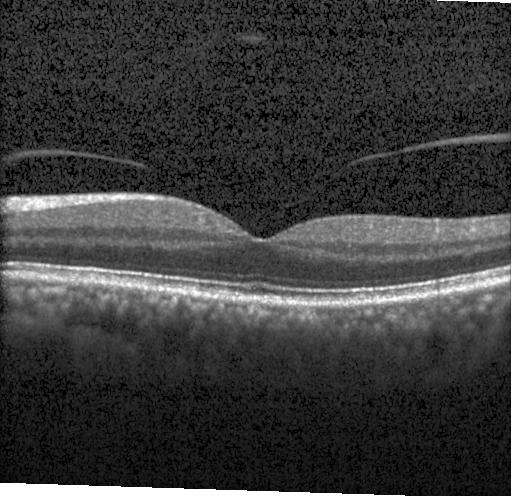

OCT line scan · spectral-domain OCT — Dx: no evidence of choroidal neovascularization, diabetic macular edema, or drusen.